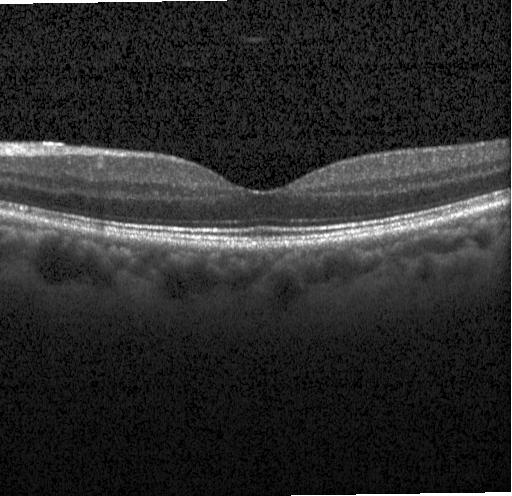 OCT B-scan. Macular OCT: no evidence of choroidal neovascularization, diabetic macular edema, or drusen.